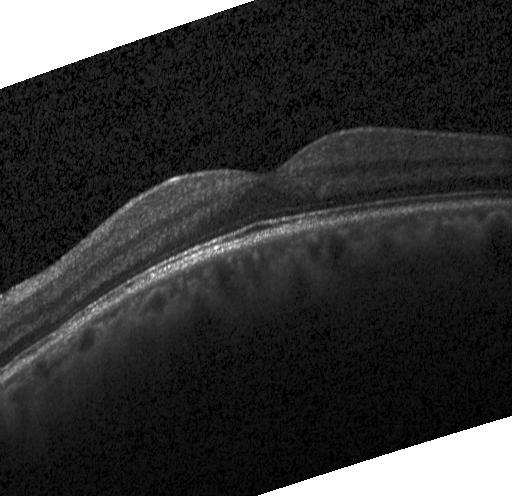
Macular scan; spectral-domain optical coherence tomography; OCT line scan. Assessment: no choroidal neovascularization, diabetic macular edema, or drusen.